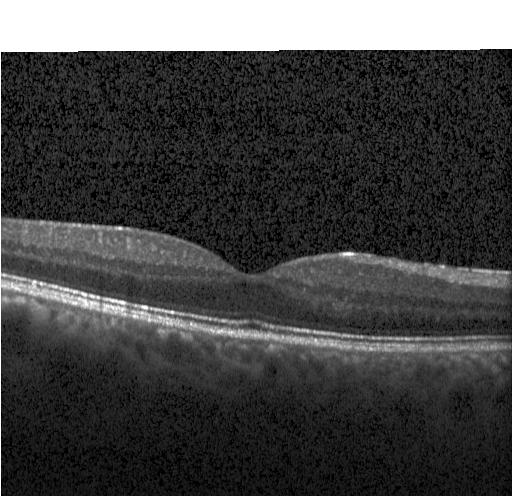 Spectral-domain optical coherence tomography; OCT B-scan; Heidelberg Spectralis OCT system — Neither choroidal neovascularization, diabetic macular edema, nor drusen.